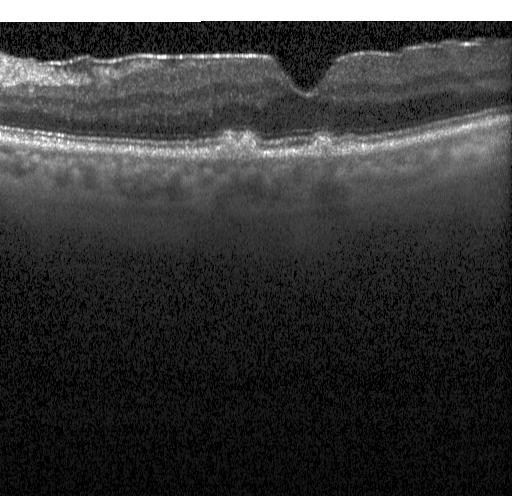 Finding: drusen.